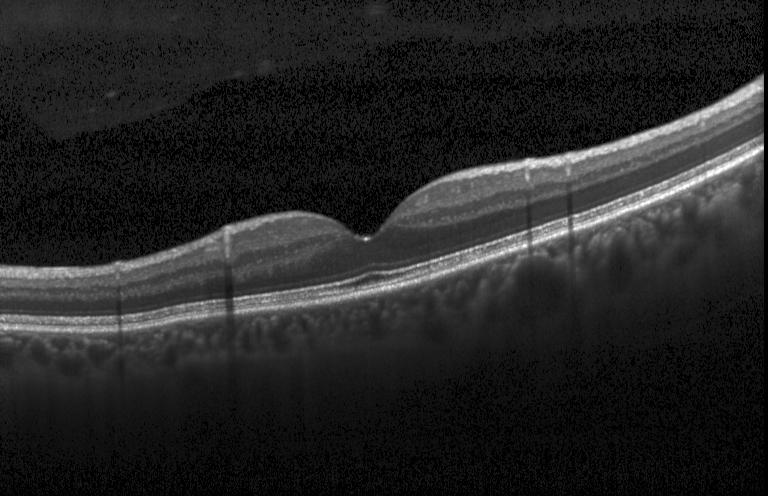

Heidelberg Spectralis, optical coherence tomography B-scan
OCT finding: no choroidal neovascularization, no diabetic macular edema, and no drusen.